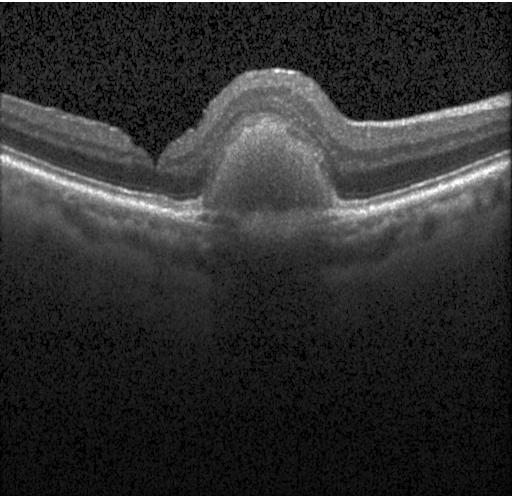
OCT line scan. Macular OCT: a choroidal neovascular membrane.